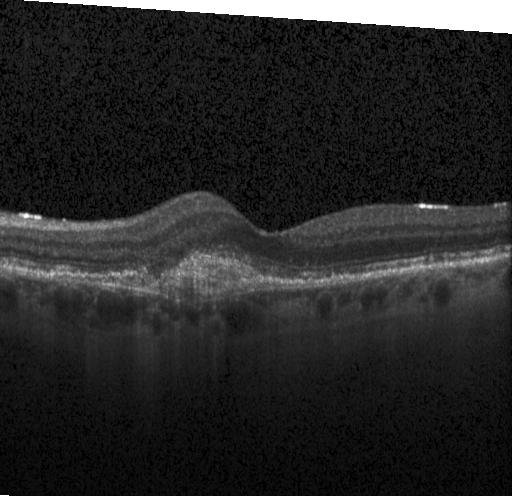
Assessment: choroidal neovascularization.